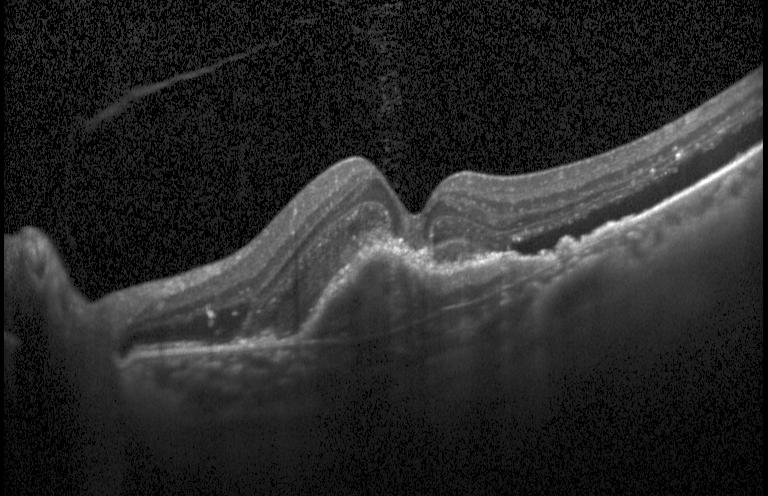

Optical coherence tomography scan. This B-scan demonstrates a choroidal neovascular membrane.